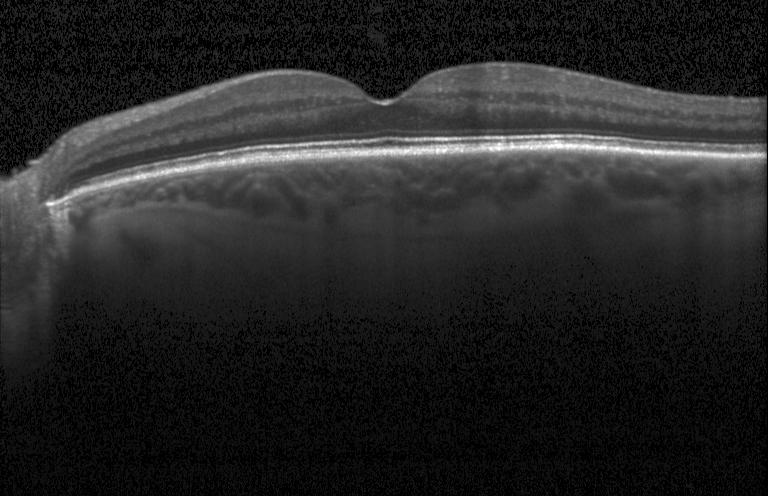

Optical coherence tomography scan.
The scan shows no CNV, DME, or drusen.